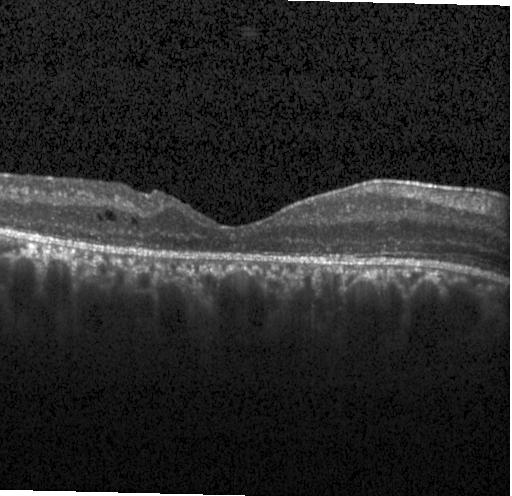

OCT line scan. Instrument: Heidelberg Spectralis. Fovea-centered. SD-OCT. Dx: diabetic macular edema.